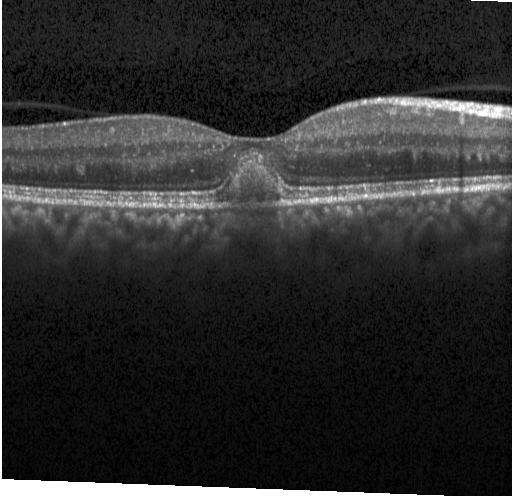
Optical coherence tomography scan
Choroidal neovascularization (CNV).